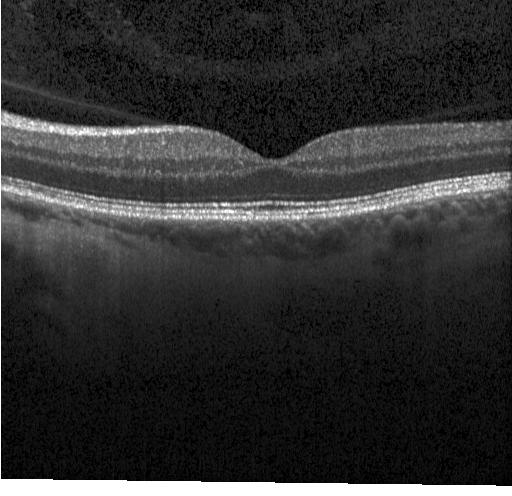
Optical coherence tomography scan · SD-OCT — The scan shows no evidence of choroidal neovascularization, diabetic macular edema, or drusen.